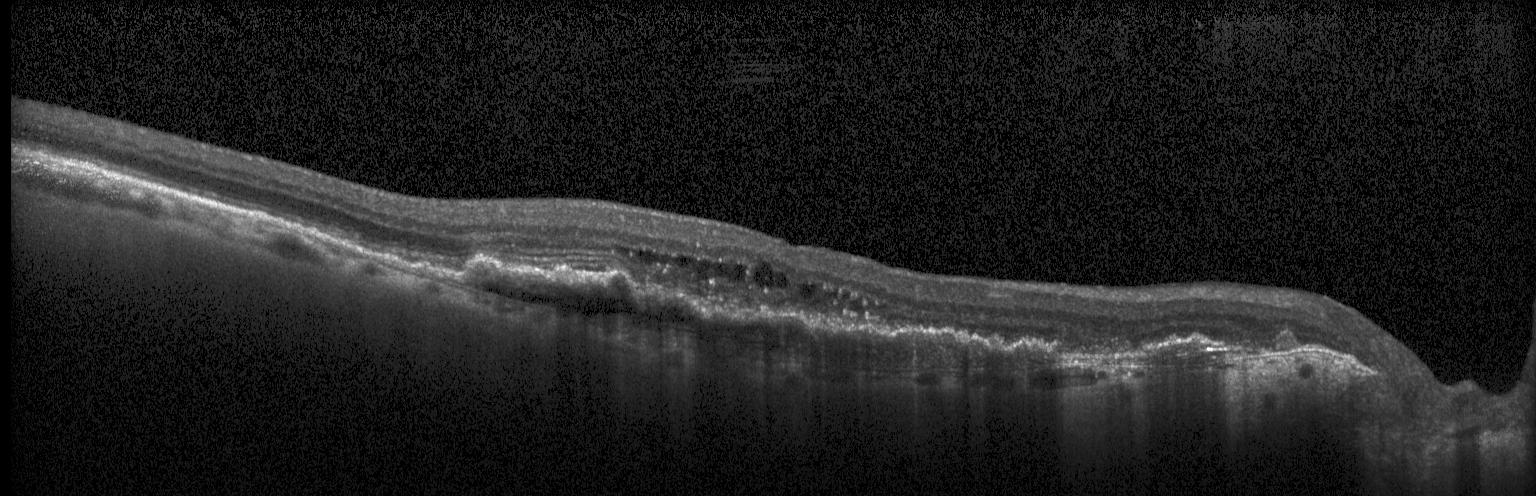

This B-scan demonstrates CNV.